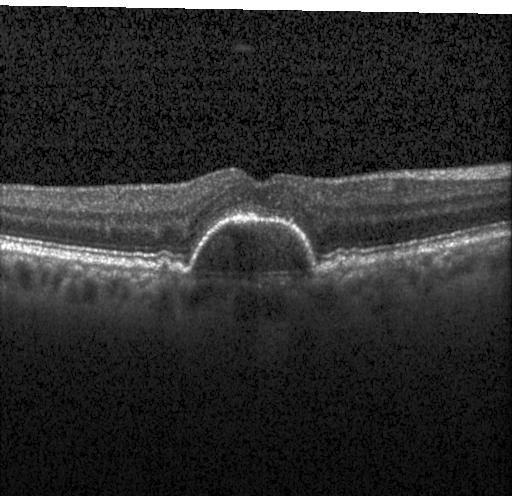
OCT line scan, spectral-domain optical coherence tomography, fovea-centered
Impression: a choroidal neovascular membrane.